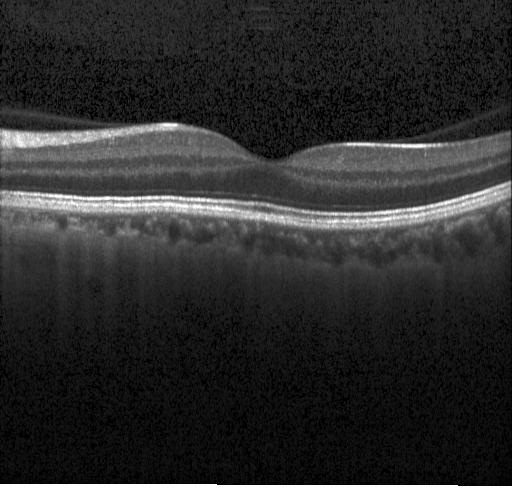
Optical coherence tomography scan, through the macula, instrument: Heidelberg Spectralis, spectral-domain optical coherence tomography — Finding: neither choroidal neovascularization, diabetic macular edema, nor drusen.